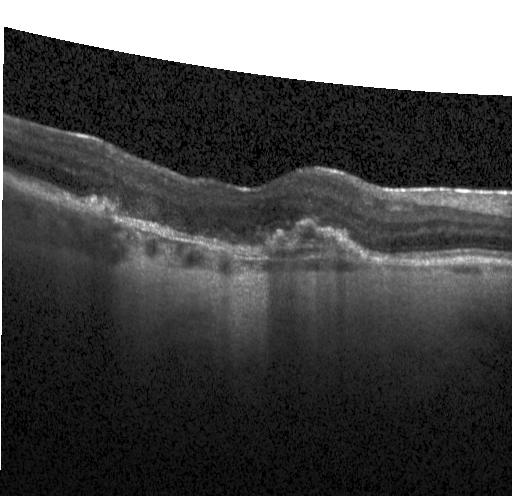

Instrument: Heidelberg Spectralis, retinal OCT B-scan, centered on the fovea, SD-OCT.
This B-scan demonstrates choroidal neovascularization.